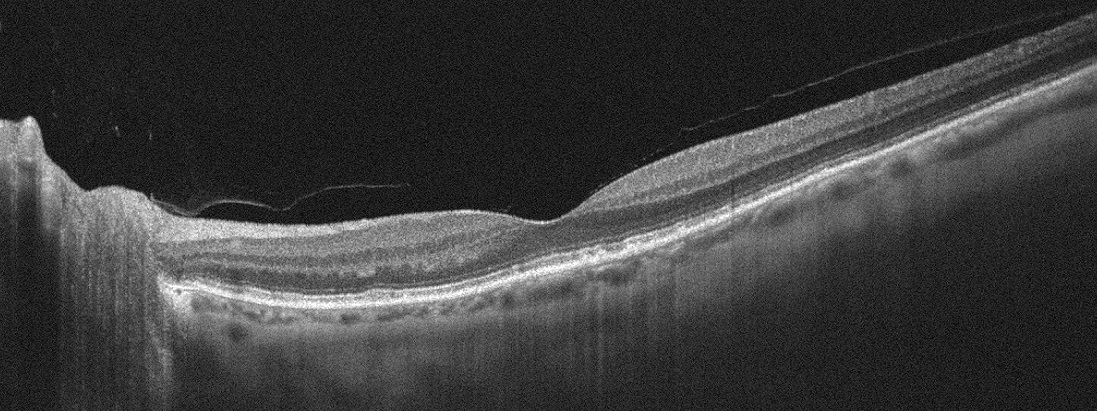 OCT line scan, through the macula. Finding: age-related macular degeneration (AMD).